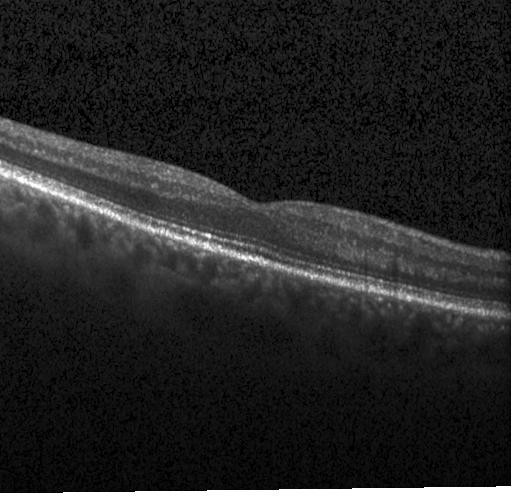

Retinal OCT cross-section showing no evidence of CNV, DME, or drusen.